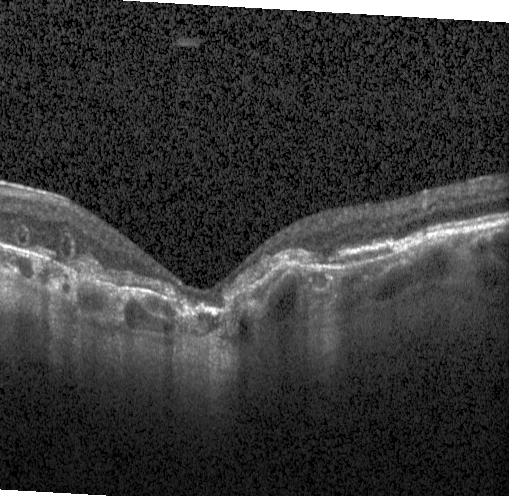

Horizontal scan through the fovea. Optical coherence tomography B-scan. Heidelberg Spectralis — This B-scan demonstrates a choroidal neovascular membrane.